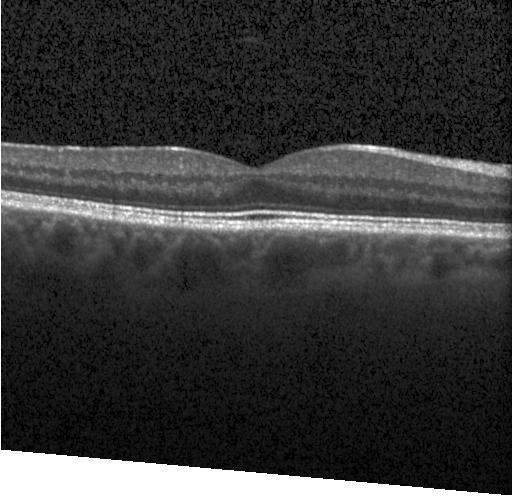

OCT scan showing no choroidal neovascularization, no diabetic macular edema, and no drusen.